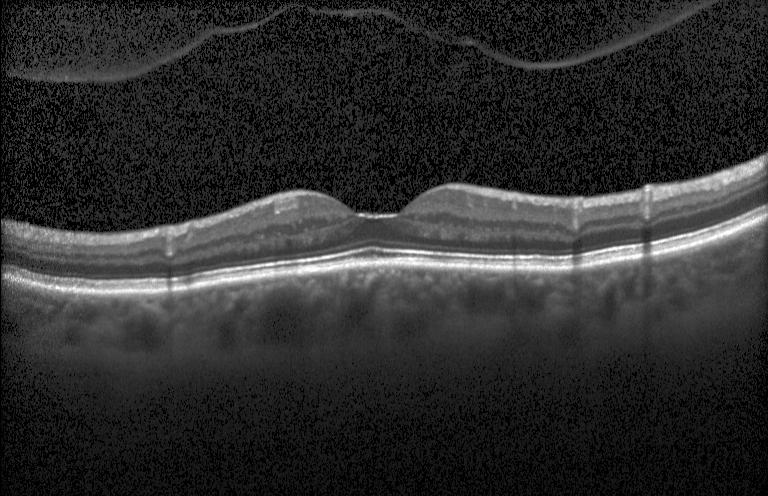

OCT finding: no evidence of choroidal neovascularization, diabetic macular edema, or drusen.